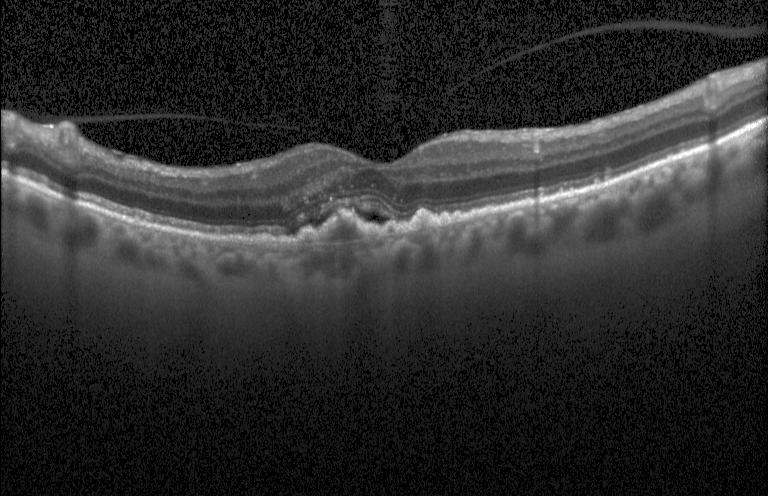

Heidelberg Spectralis · horizontal scan through the fovea · retinal OCT cross-section
Diagnosis: CNV.